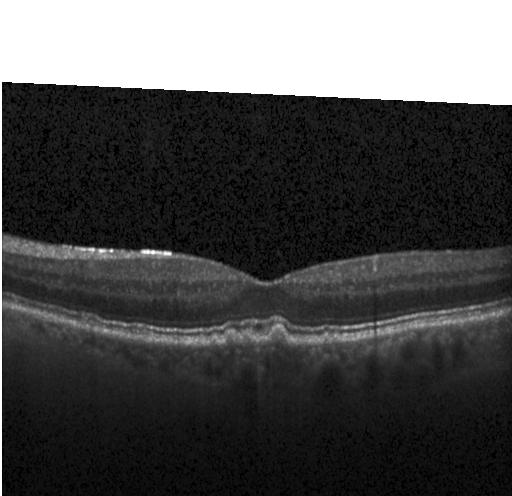
OCT B-scan showing drusen.